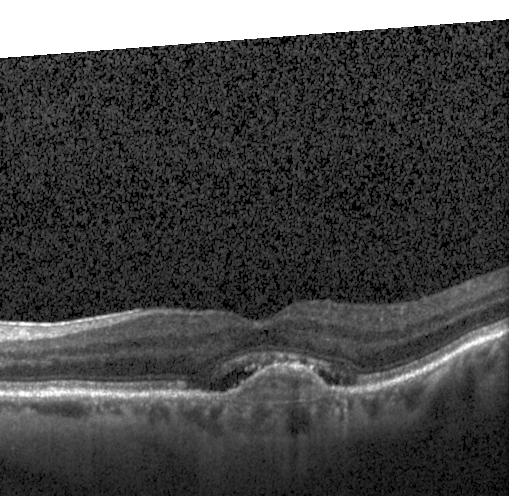
OCT scan showing choroidal neovascularization.